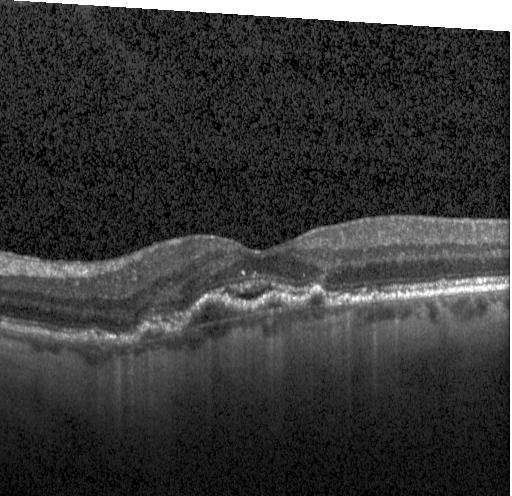
OCT line scan; spectral-domain OCT — Diagnosis: a choroidal neovascular membrane.